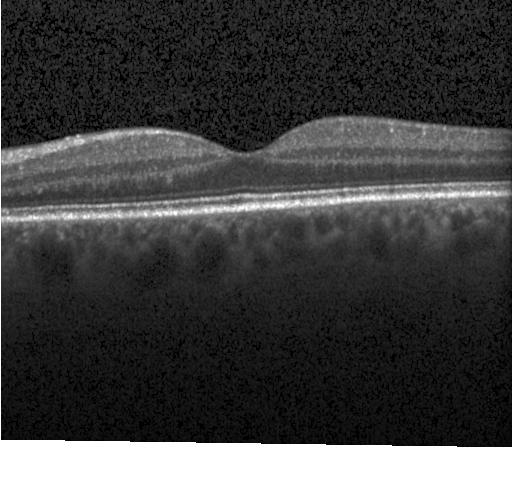

Finding: no evidence of choroidal neovascularization, diabetic macular edema, or drusen.